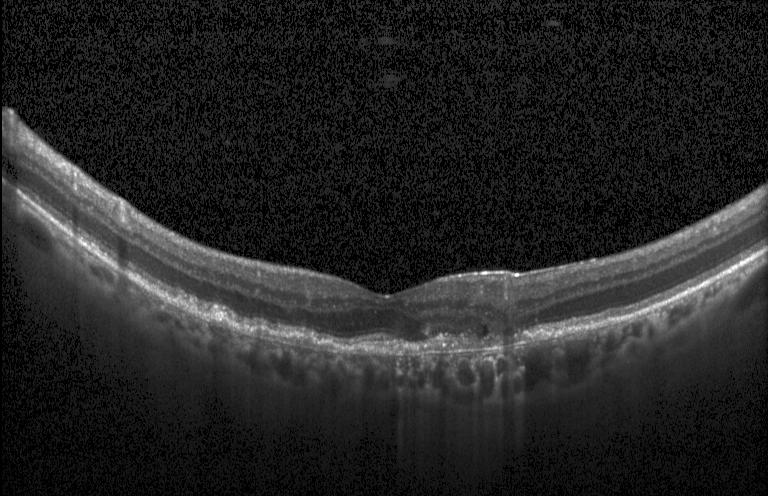

Spectral-domain OCT B-scan: a choroidal neovascular membrane.